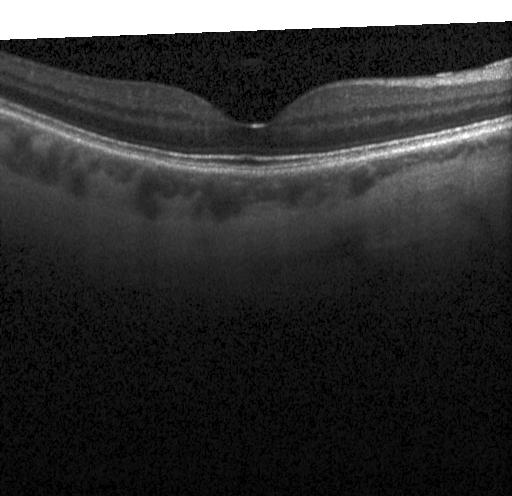 Macular OCT: neither CNV, DME, nor drusen.